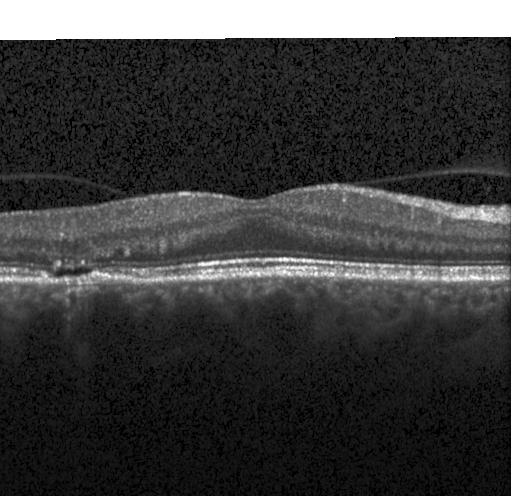 Macular OCT: a choroidal neovascular membrane.